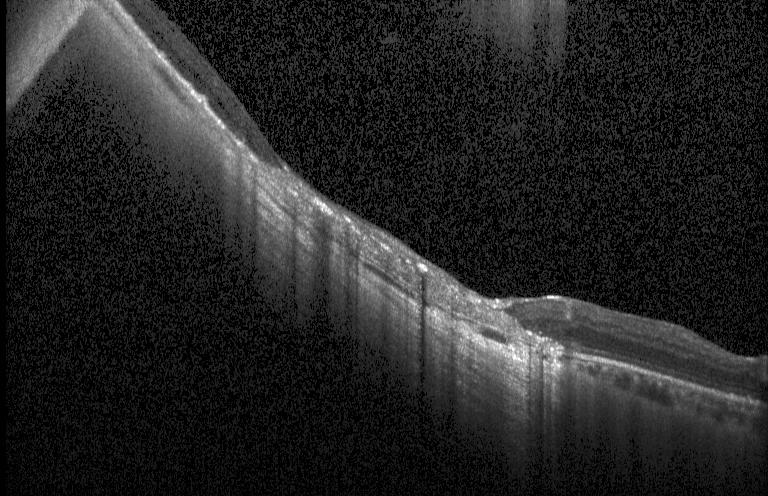 SD-OCT. Centered on the fovea. OCT line scan — Diagnosis: choroidal neovascularization.